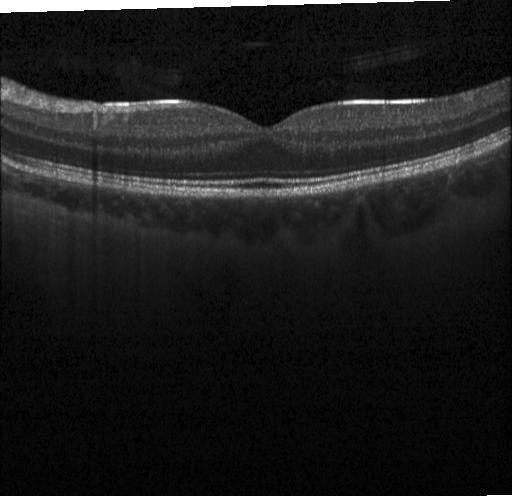
Diagnosis: neither choroidal neovascularization, diabetic macular edema, nor drusen.